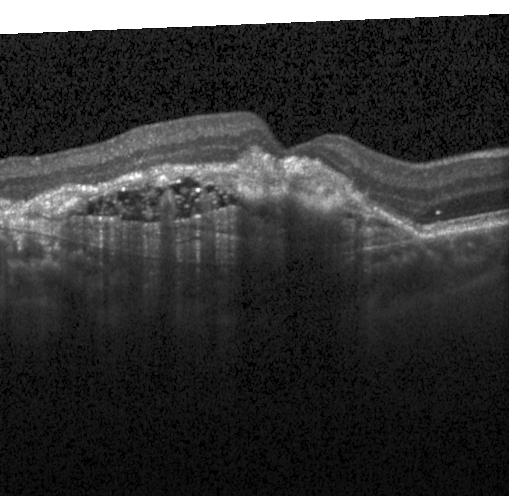

OCT B-scan.
Assessment: choroidal neovascularization.